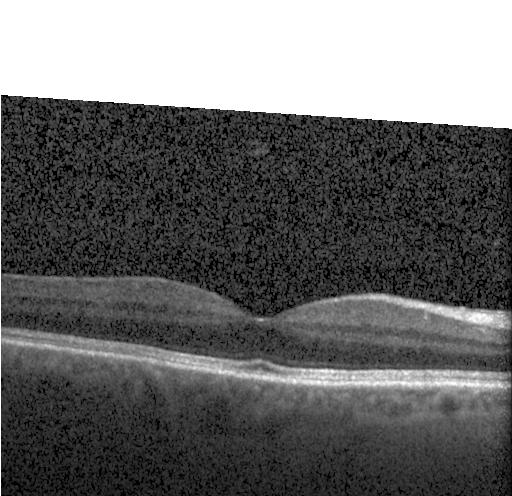 Diagnosis: no CNV, no DME, and no drusen.